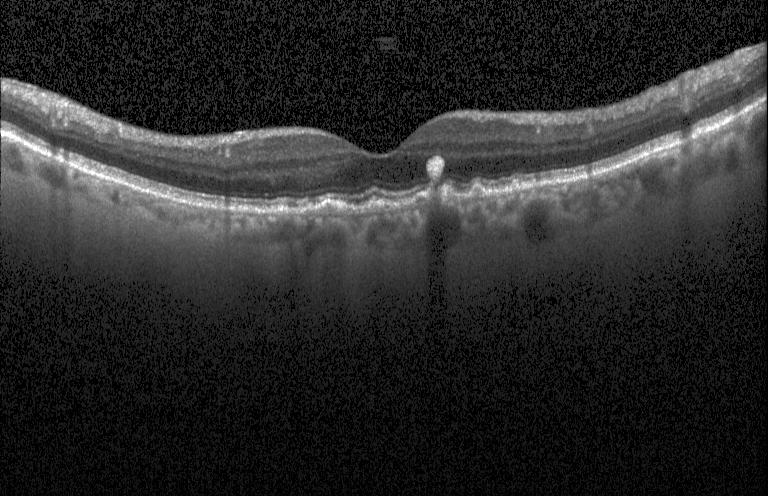 SD-OCT, optical coherence tomography B-scan, macular scan, instrument: Heidelberg Spectralis
Assessment: drusen.